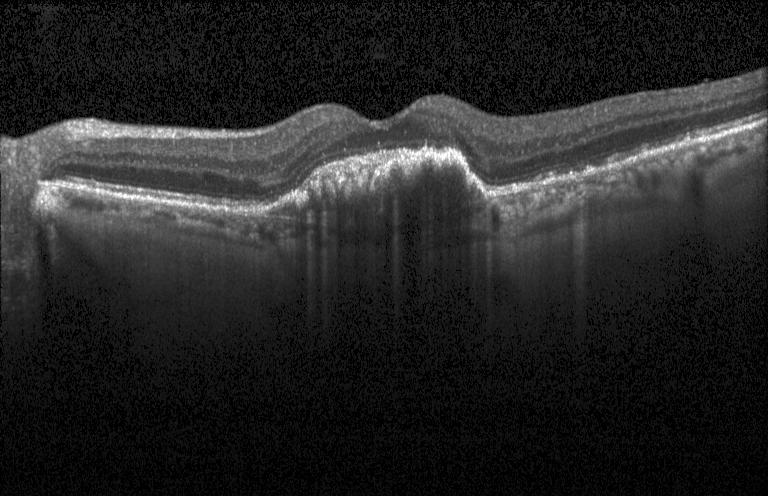

OCT finding: a choroidal neovascular membrane.